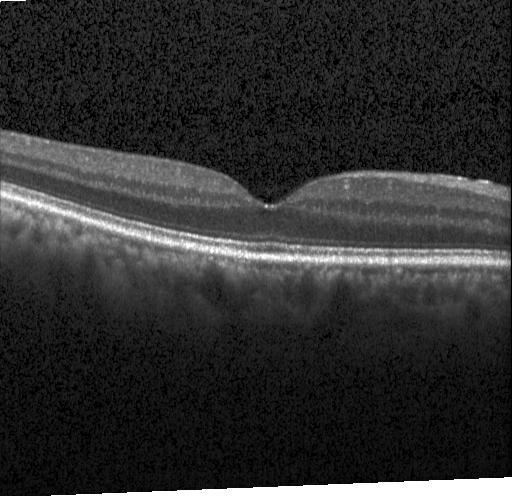
Retinal OCT B-scan. Through the macula
Finding: neither CNV, DME, nor drusen.